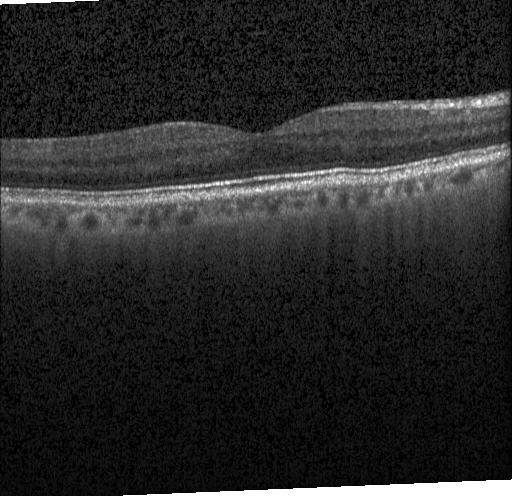
Through the macula. SD-OCT. Heidelberg Spectralis OCT system. Optical coherence tomography B-scan
Assessment: no choroidal neovascularization, diabetic macular edema, or drusen.